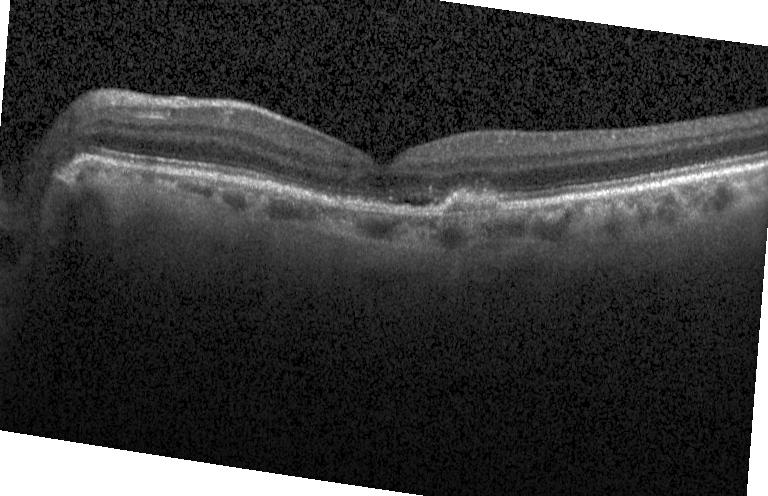 OCT finding: choroidal neovascularization (CNV).